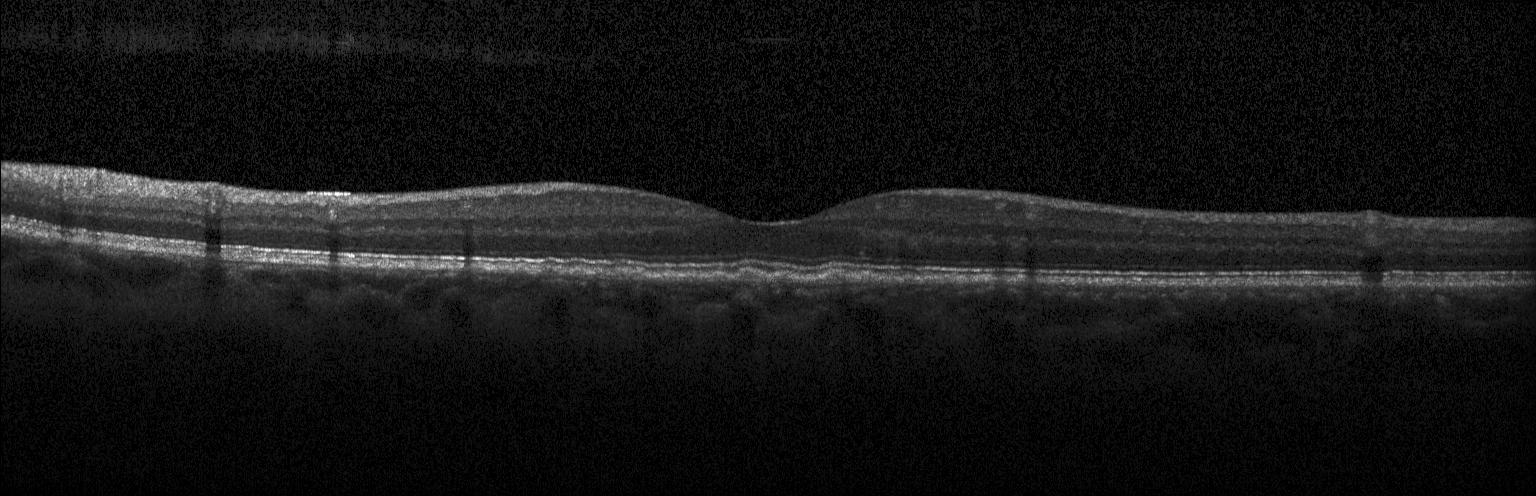

OCT finding: multiple drusen.